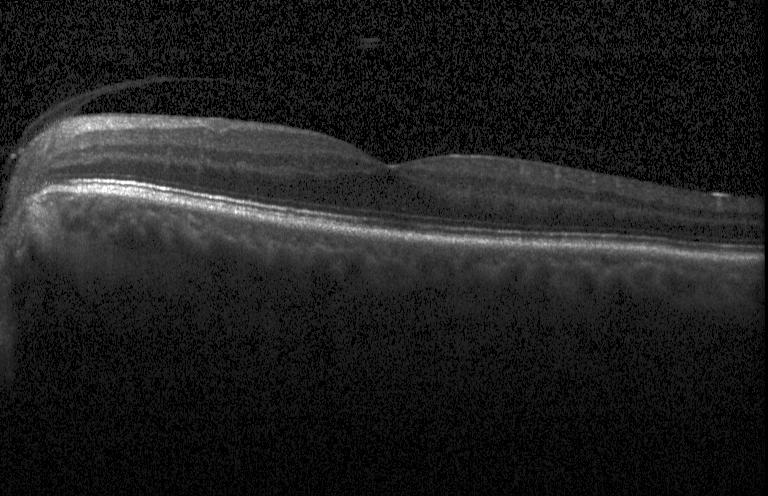

Optical coherence tomography B-scan · spectral-domain optical coherence tomography — Finding: no evidence of choroidal neovascularization, diabetic macular edema, or drusen.